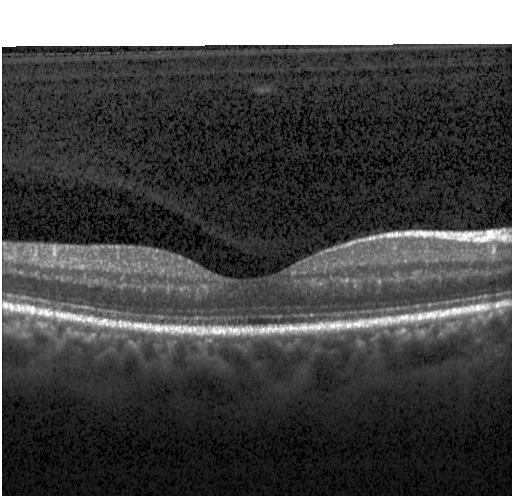 This B-scan demonstrates neither choroidal neovascularization, diabetic macular edema, nor drusen.